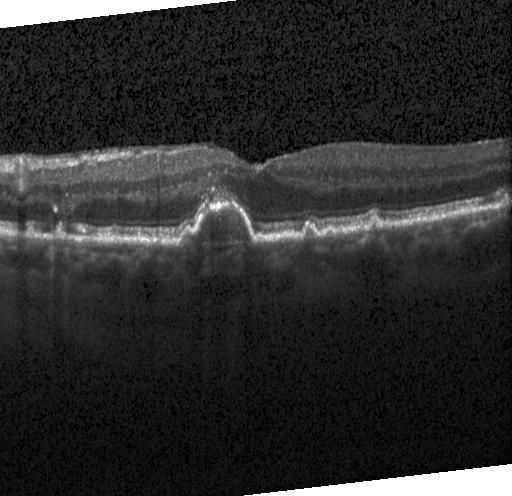
OCT scan showing drusen.